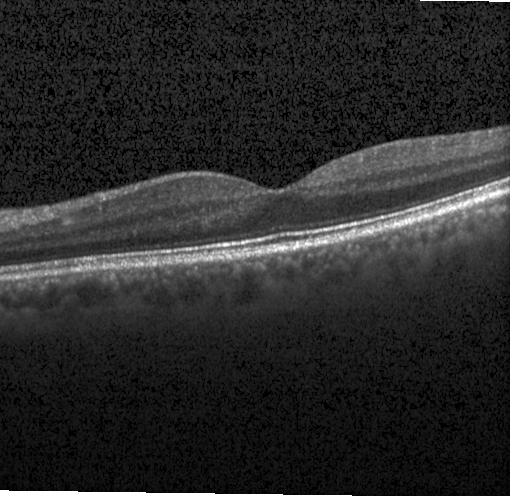
Spectral-domain OCT; macular scan; OCT line scan; Heidelberg Spectralis OCT system — This B-scan demonstrates no CNV, no DME, and no drusen.